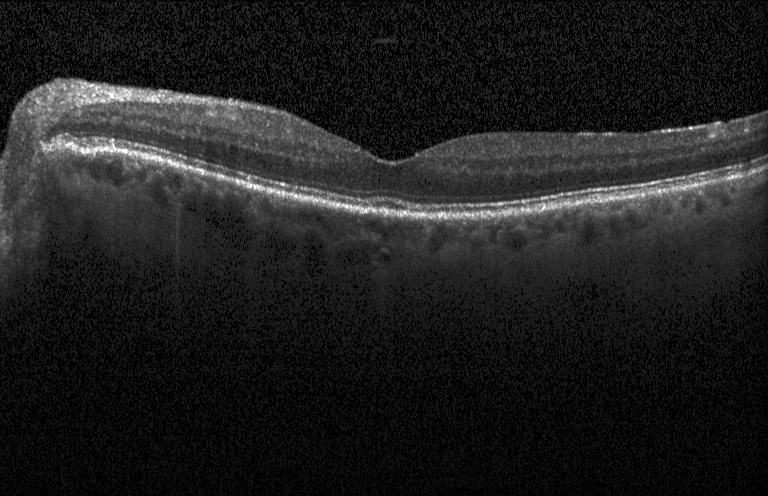
Finding: neither choroidal neovascularization, diabetic macular edema, nor drusen.